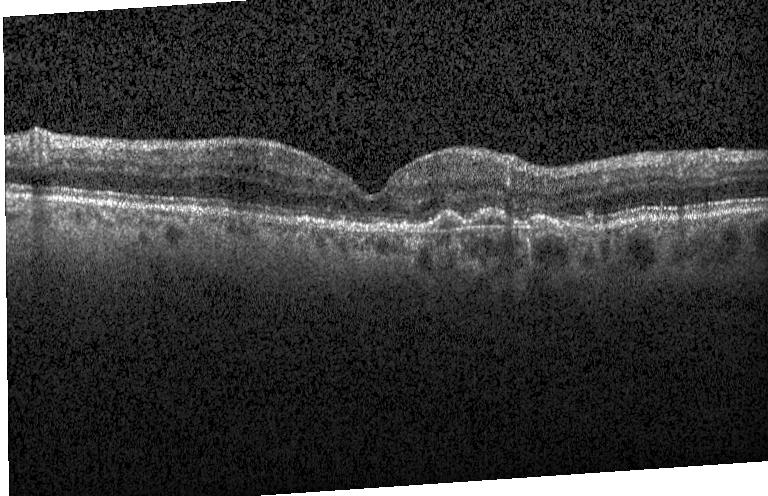 Finding: a choroidal neovascular membrane.